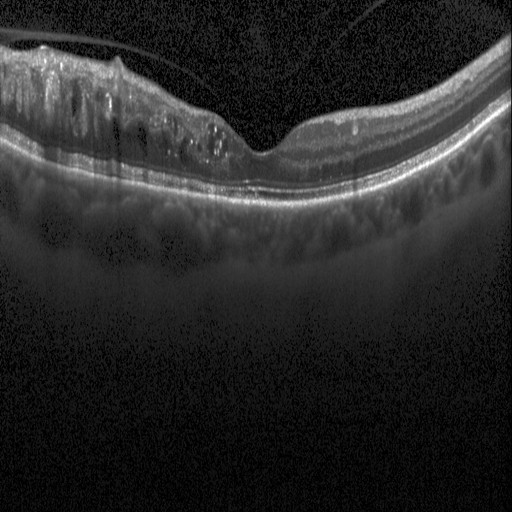
Horizontal scan through the fovea; retinal OCT B-scan.
Finding: DME.